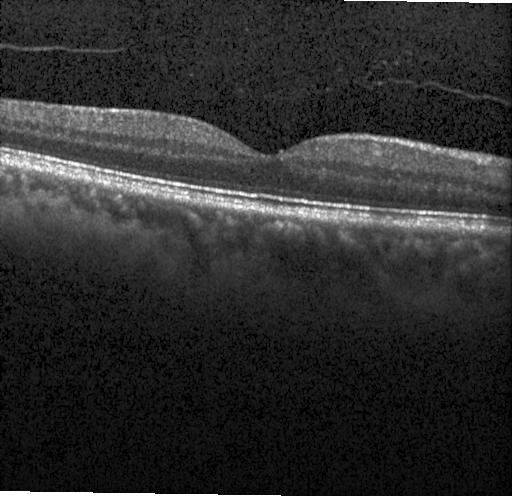
Optical coherence tomography scan; instrument: Heidelberg Spectralis
Diagnosis: no choroidal neovascularization, diabetic macular edema, or drusen.